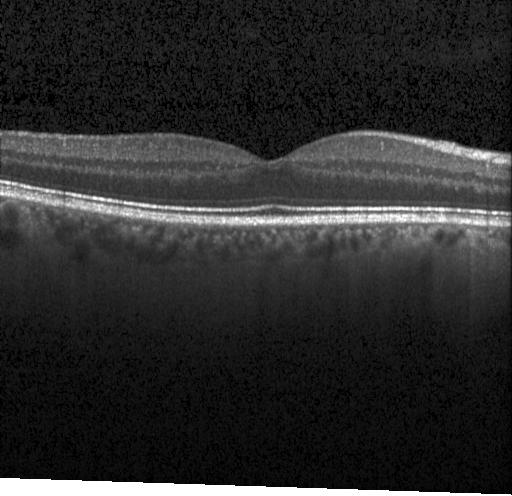

Fovea-centered. SD-OCT. OCT line scan
The scan shows neither choroidal neovascularization, diabetic macular edema, nor drusen.